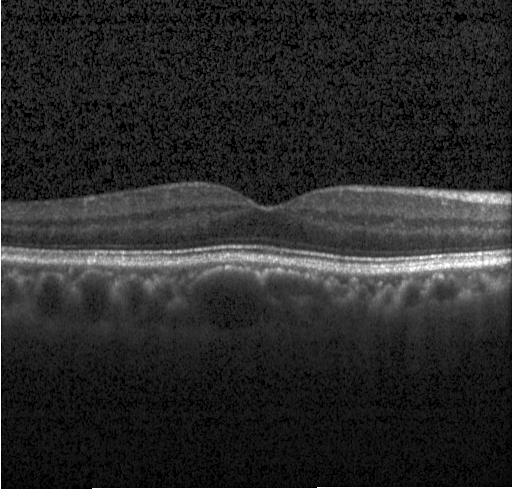
Centered on the fovea; OCT B-scan — Diagnosis: no evidence of choroidal neovascularization, diabetic macular edema, or drusen.